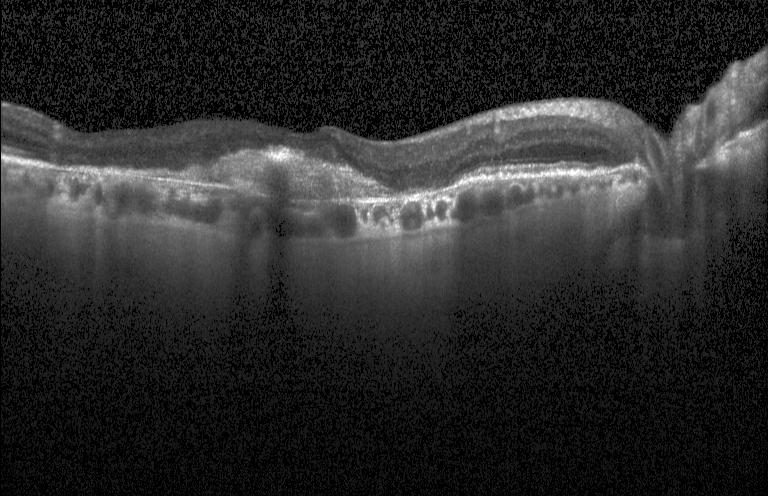
OCT scan showing a choroidal neovascular membrane.